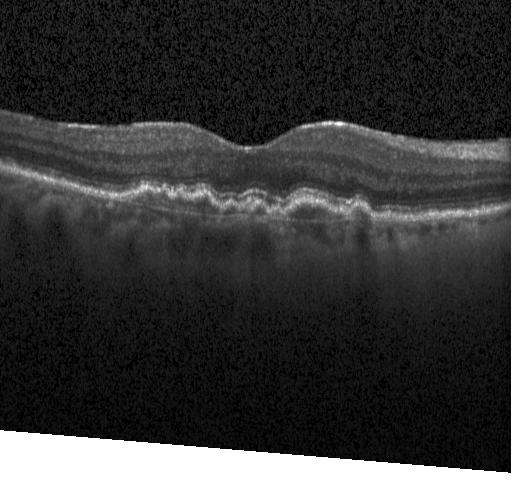 Spectral-domain OCT. Fovea-centered. Acquired on a Heidelberg Spectralis. Retinal OCT cross-section
Finding: CNV.